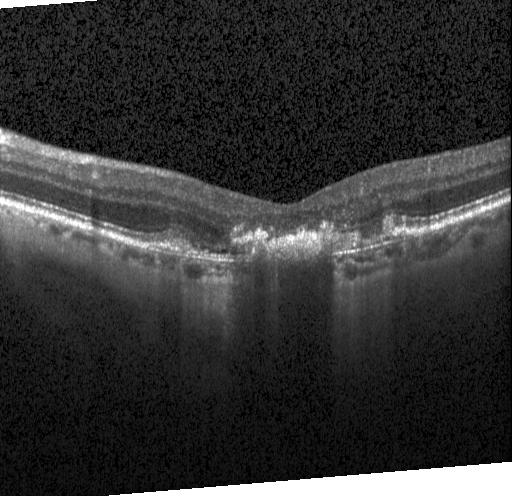

Finding: a choroidal neovascular membrane.